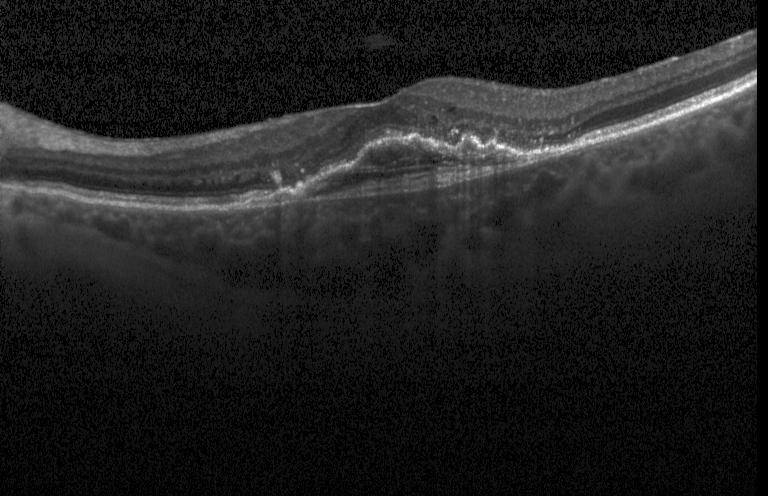

OCT line scan. Assessment: choroidal neovascularization.